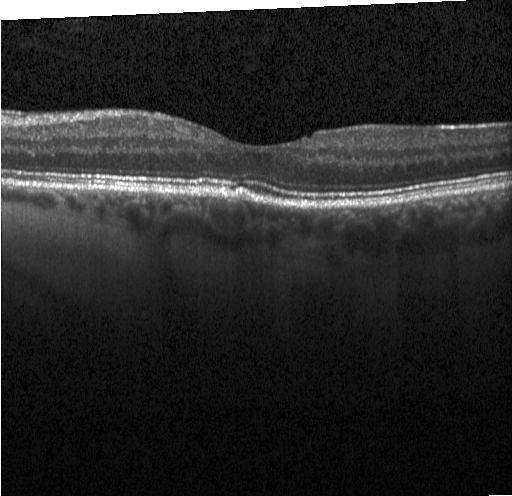

Optical coherence tomography B-scan
OCT finding: drusen.